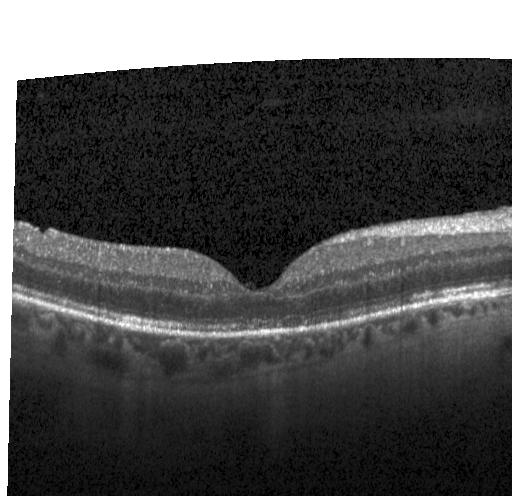 Spectral-domain optical coherence tomography. Instrument: Heidelberg Spectralis. Optical coherence tomography B-scan. OCT finding: no CNV, DME, or drusen.